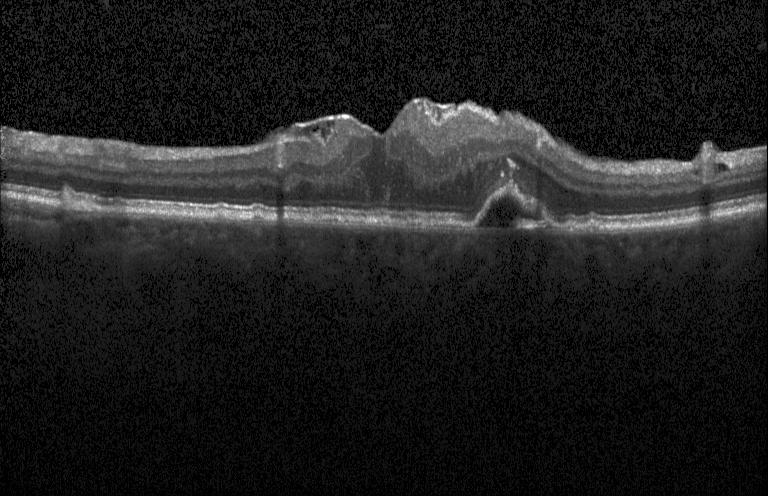

OCT line scan, spectral-domain OCT, Heidelberg Spectralis, fovea-centered. OCT finding: CNV.